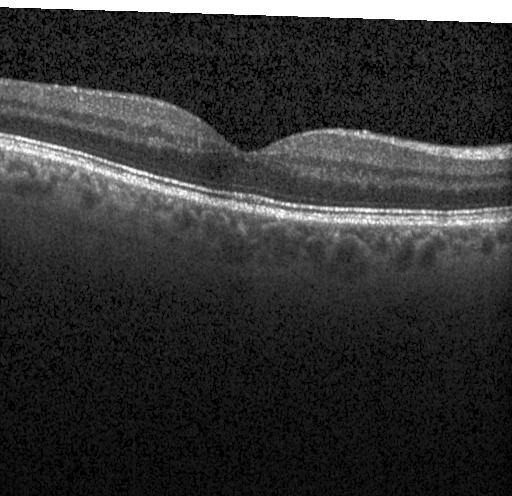
OCT line scan — This B-scan demonstrates no choroidal neovascularization, no diabetic macular edema, and no drusen.